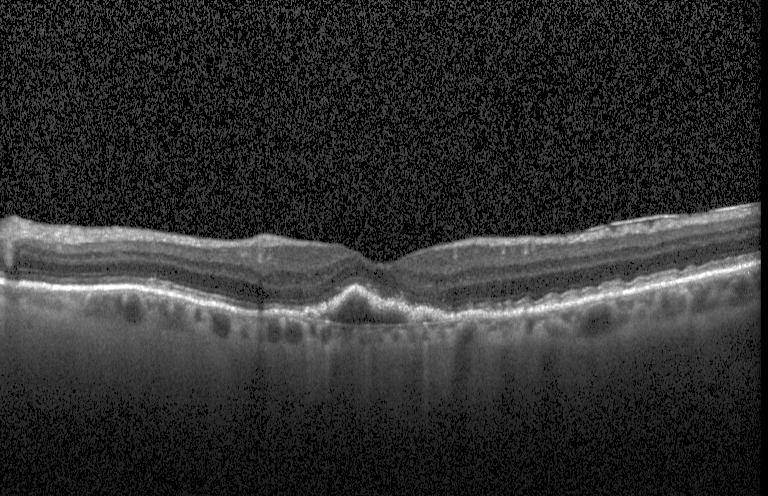

Optical coherence tomography B-scan
Dx: choroidal neovascularization.